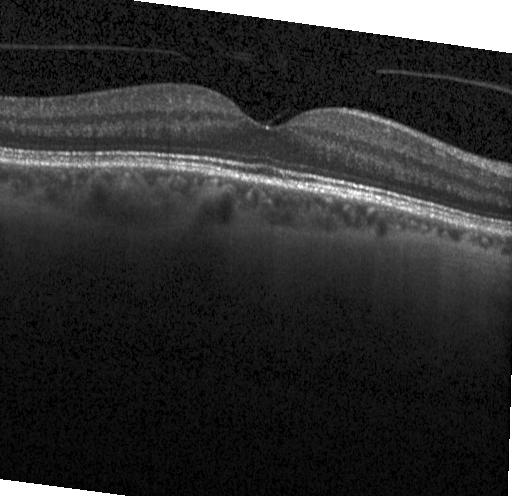
Impression: no CNV, no DME, and no drusen.